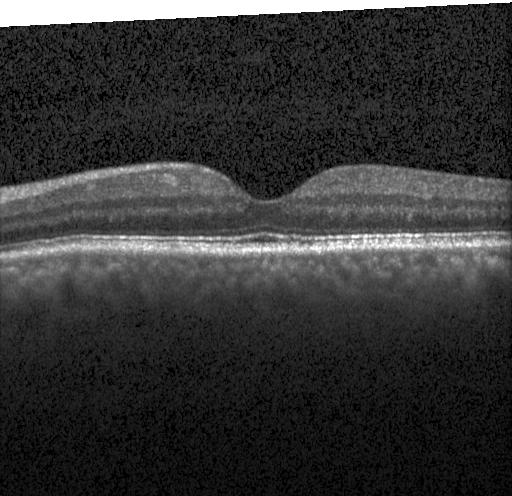

Optical coherence tomography B-scan
Impression: no CNV, no DME, and no drusen.